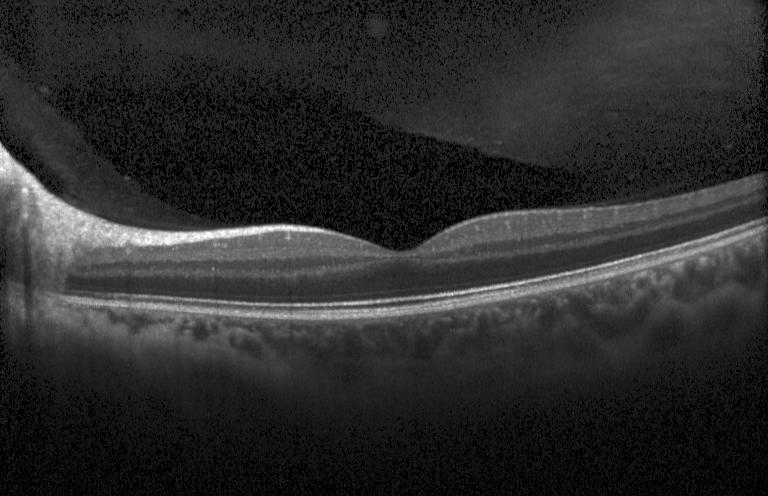
Fovea-centered. OCT line scan.
No choroidal neovascularization, diabetic macular edema, or drusen.